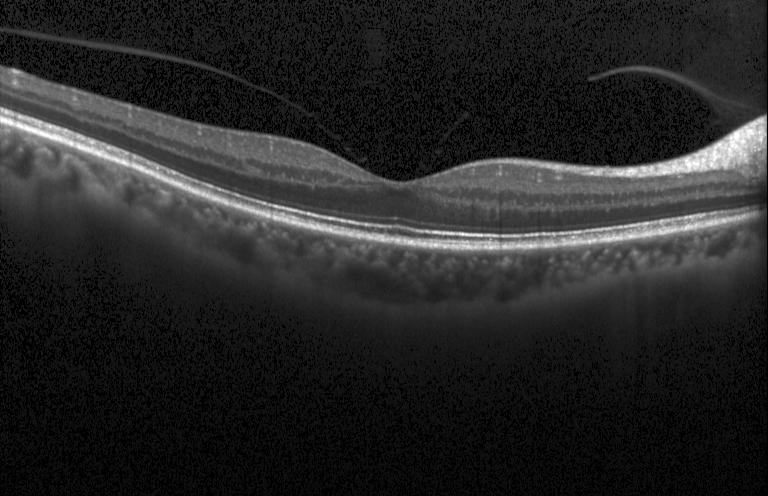

Macular OCT: no choroidal neovascularization, diabetic macular edema, or drusen.